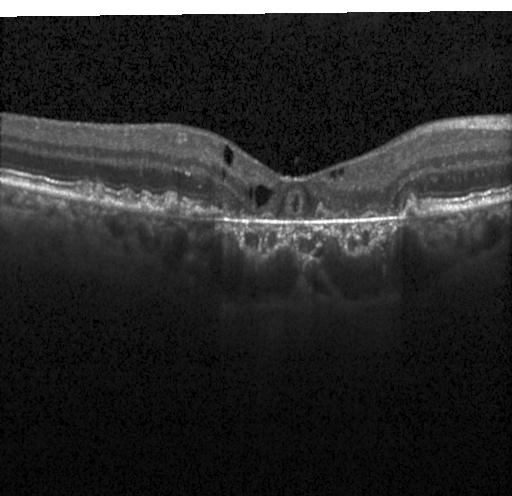
Heidelberg Spectralis, retinal OCT B-scan.
This B-scan demonstrates a choroidal neovascular membrane.